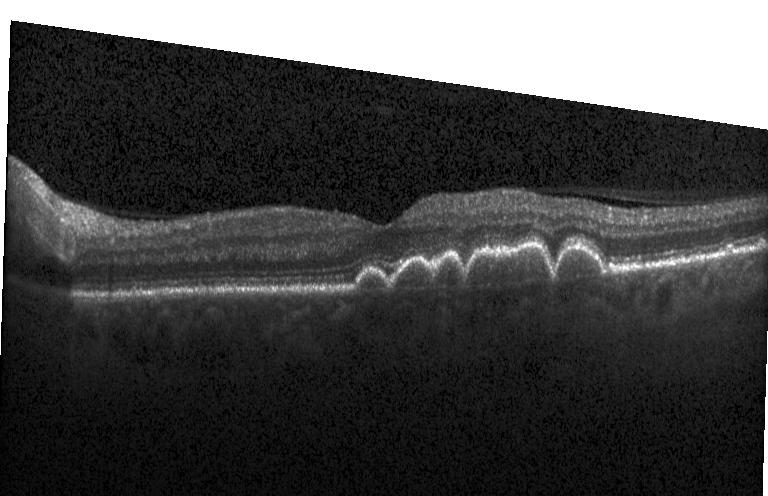

Optical coherence tomography B-scan, instrument: Heidelberg Spectralis.
Impression: drusen.